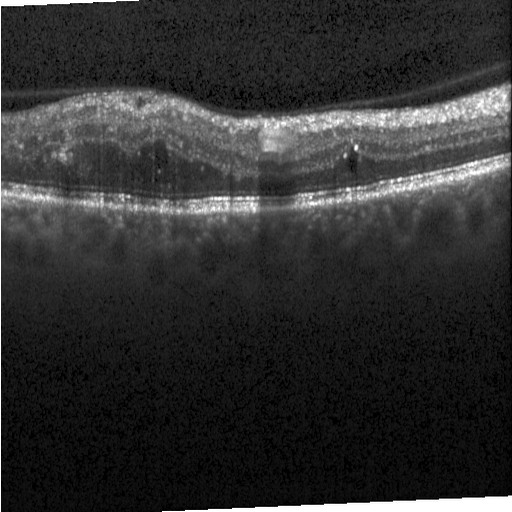 Heidelberg Spectralis OCT system. Retinal OCT B-scan. Spectral-domain OCT. Horizontal scan through the fovea — Impression: DME.